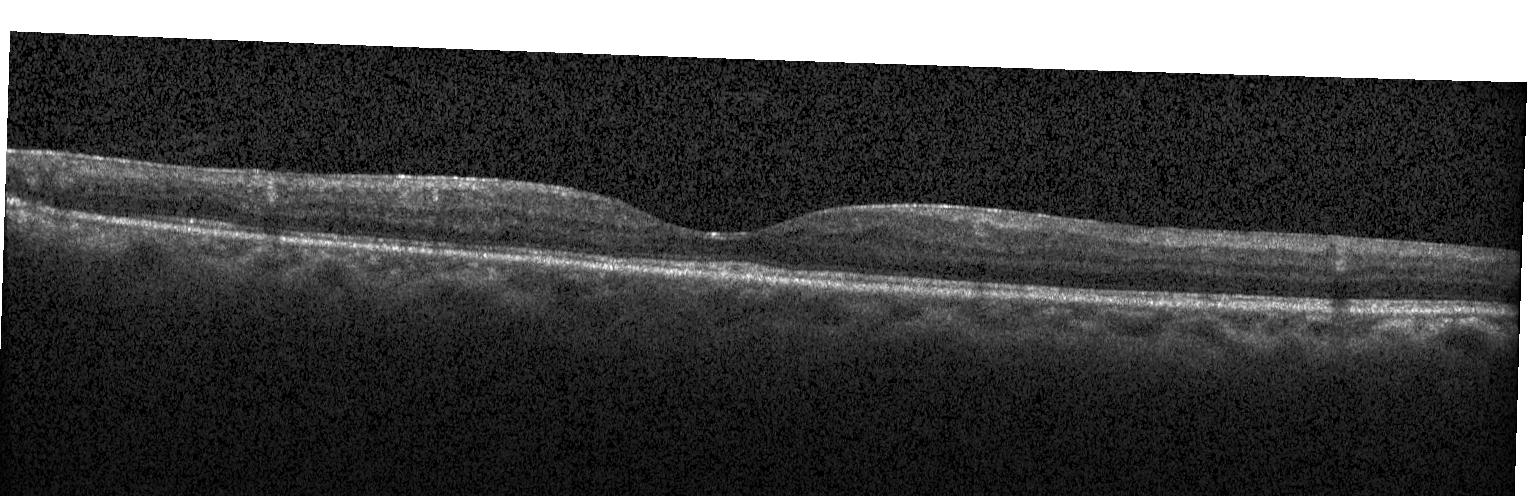
Centered on the fovea; acquired on a Heidelberg Spectralis; retinal OCT cross-section.
This B-scan demonstrates no evidence of CNV, DME, or drusen.